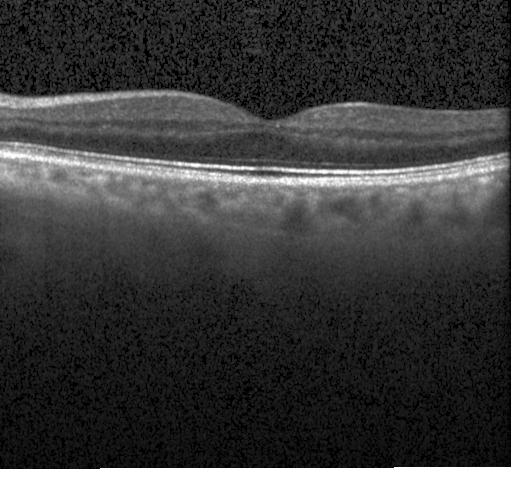
Heidelberg Spectralis OCT system · spectral-domain optical coherence tomography · optical coherence tomography B-scan.
Finding: neither choroidal neovascularization, diabetic macular edema, nor drusen.